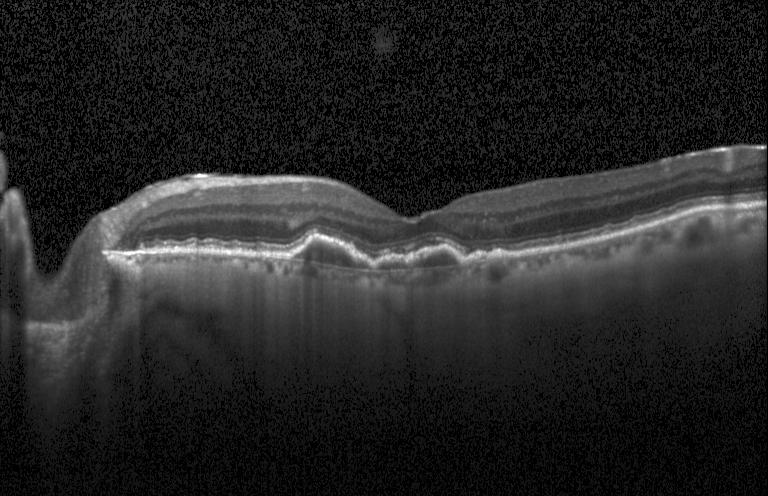
OCT B-scan. The scan shows a choroidal neovascular membrane.